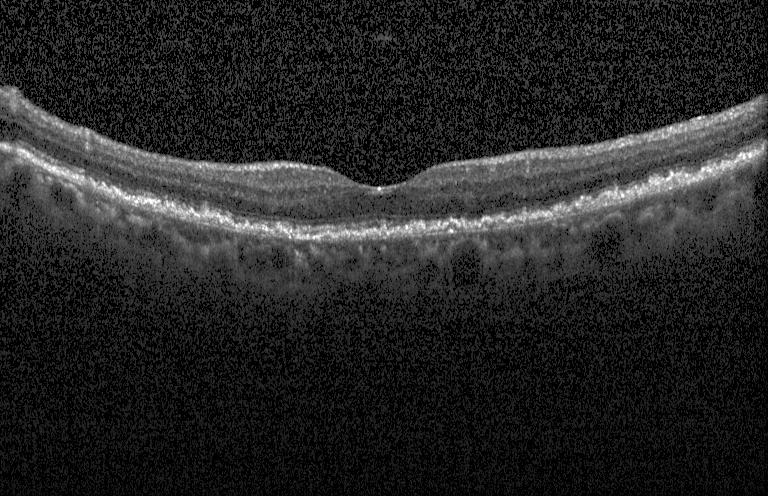
The scan shows drusen.